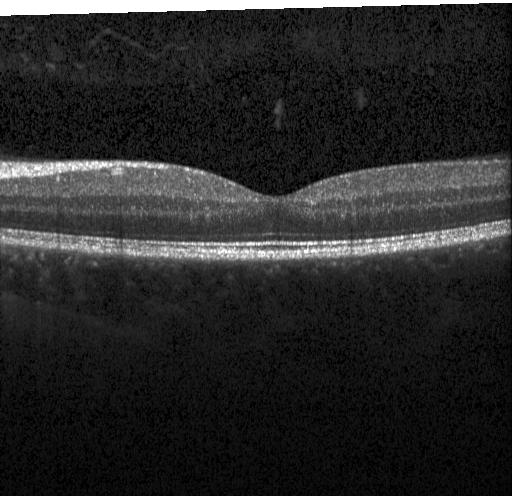

Finding: no choroidal neovascularization, diabetic macular edema, or drusen.